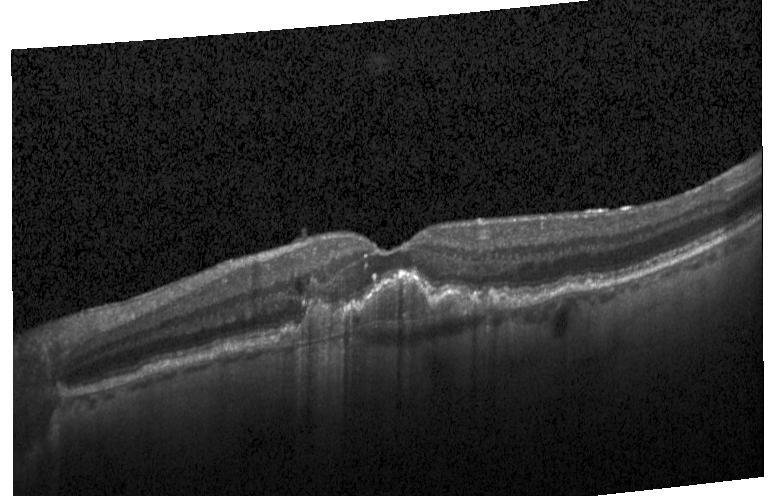
Retinal OCT cross-section. Diagnosis: a choroidal neovascular membrane.